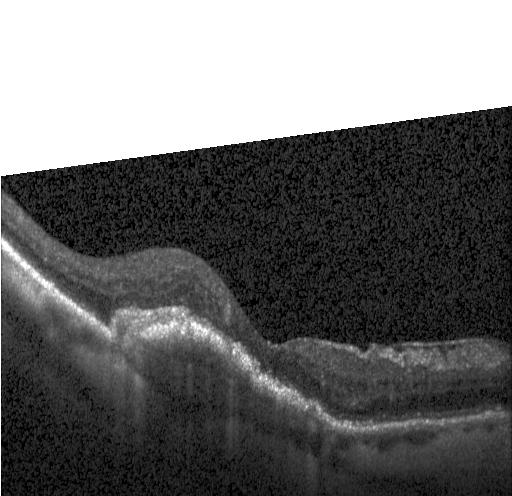

Optical coherence tomography B-scan, Heidelberg Spectralis, centered on the fovea
Impression: choroidal neovascularization (CNV).